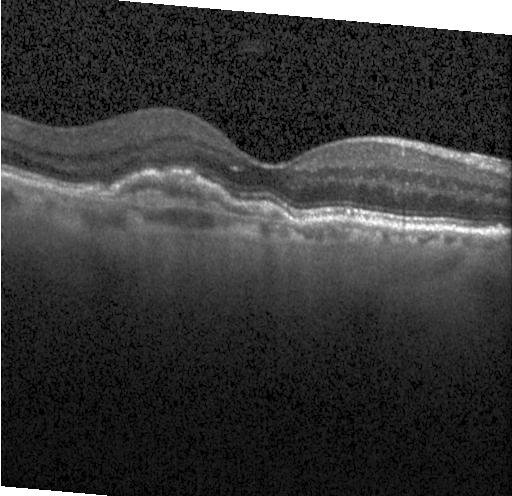

Retinal OCT cross-section · Heidelberg Spectralis OCT system · fovea-centered.
This B-scan demonstrates a choroidal neovascular membrane.